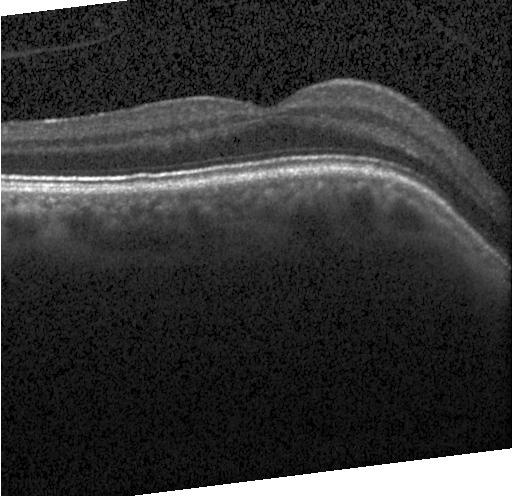
OCT line scan · through the macula · acquired on a Heidelberg Spectralis · spectral-domain OCT — This B-scan demonstrates no CNV, no DME, and no drusen.